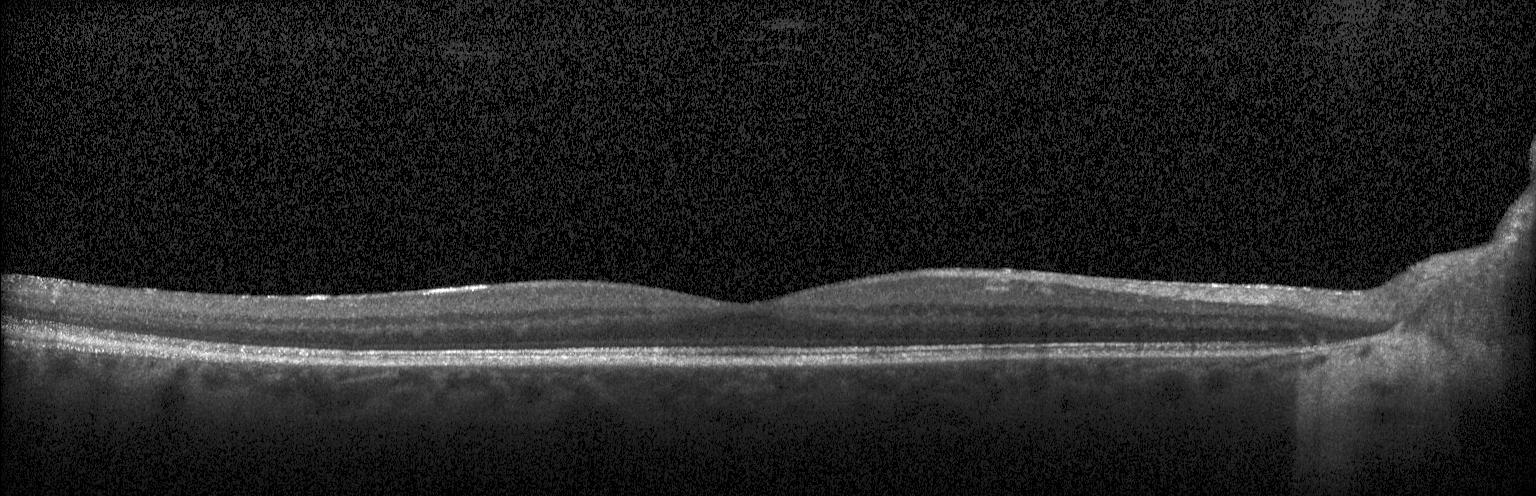
Retinal OCT B-scan, Heidelberg Spectralis OCT system — Impression: no evidence of CNV, DME, or drusen.